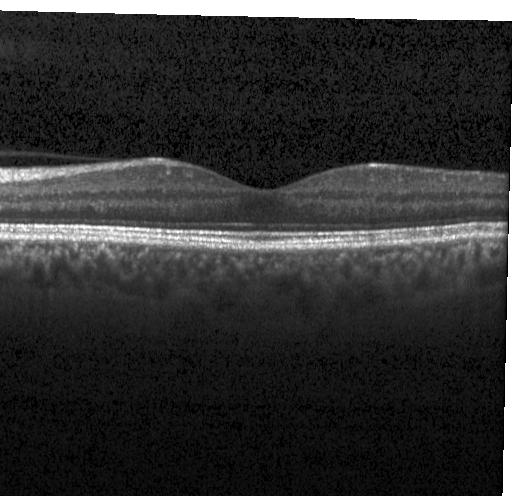

Optical coherence tomography B-scan. Heidelberg Spectralis OCT system
Diagnosis: neither CNV, DME, nor drusen.